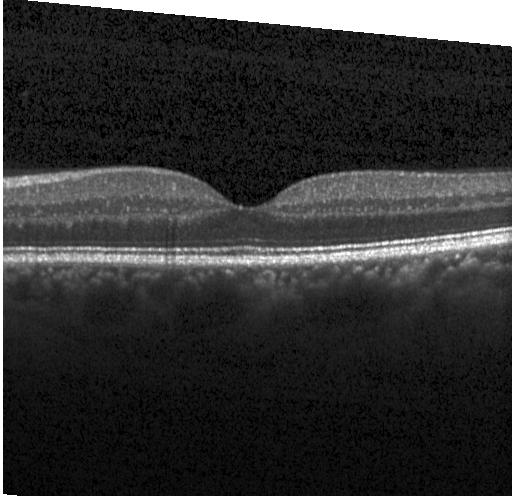
OCT line scan. Heidelberg Spectralis. Macular scan — OCT finding: no choroidal neovascularization, no diabetic macular edema, and no drusen.